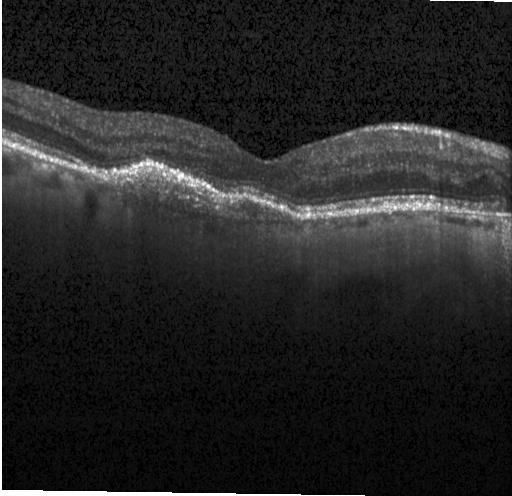

Optical coherence tomography B-scan
Finding: a choroidal neovascular membrane.